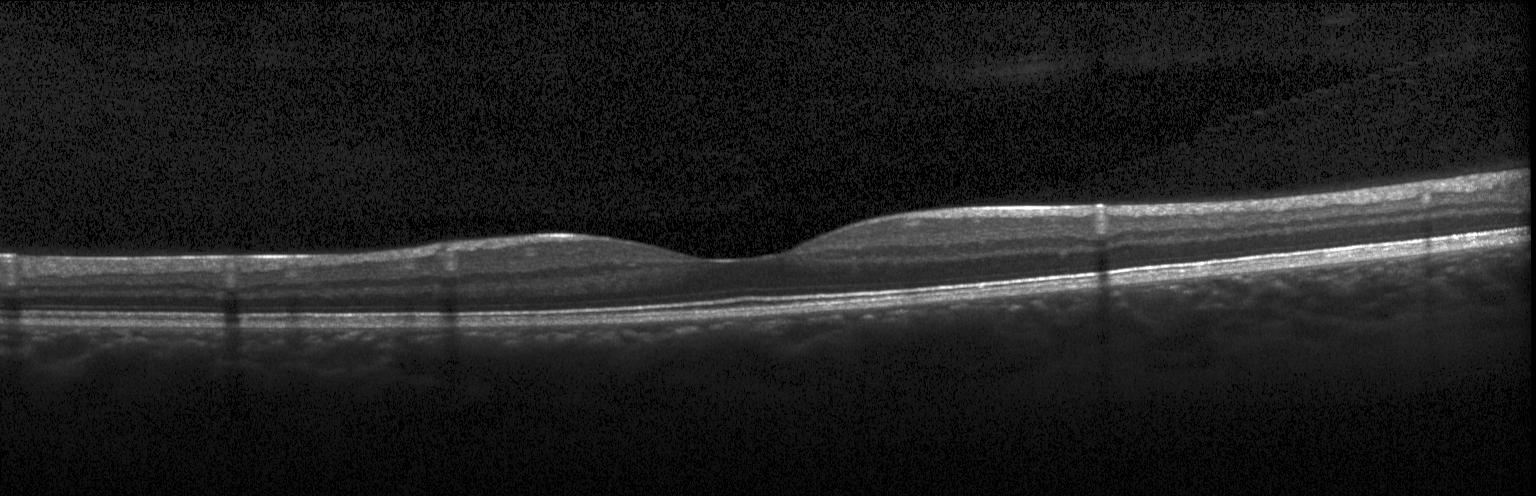
Impression: no evidence of choroidal neovascularization, diabetic macular edema, or drusen.